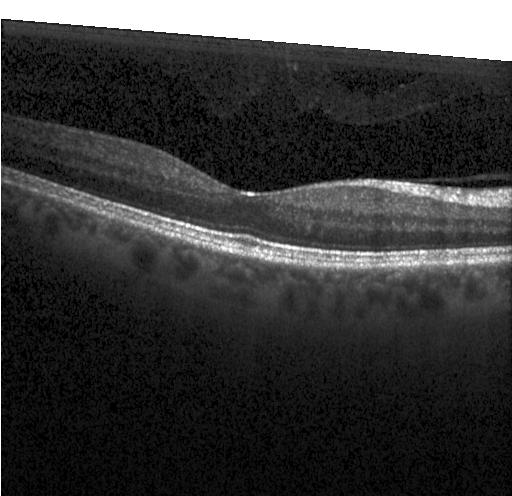

OCT line scan
OCT finding: no evidence of choroidal neovascularization, diabetic macular edema, or drusen.